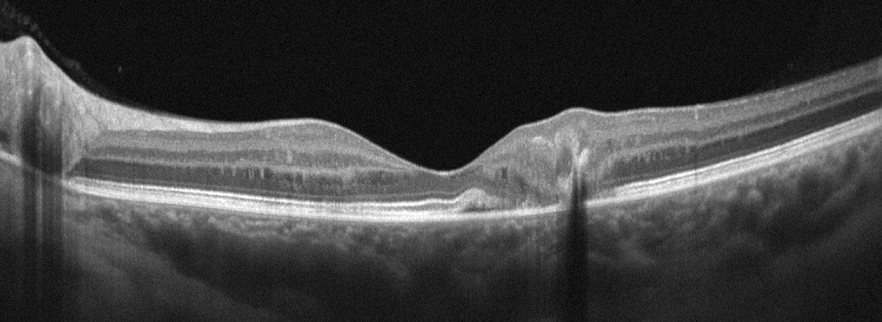

OS · OCT line scan.
Macular OCT: age-related macular degeneration (AMD).